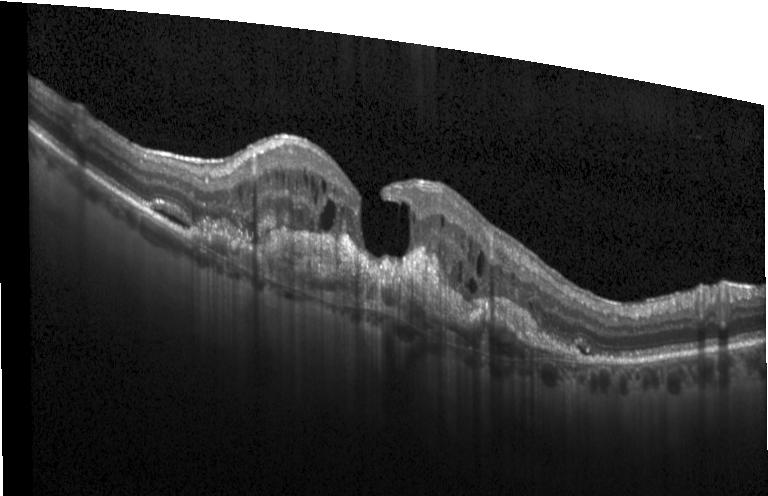 Heidelberg Spectralis OCT system · OCT line scan · spectral-domain optical coherence tomography · fovea-centered — This B-scan demonstrates a choroidal neovascular membrane.